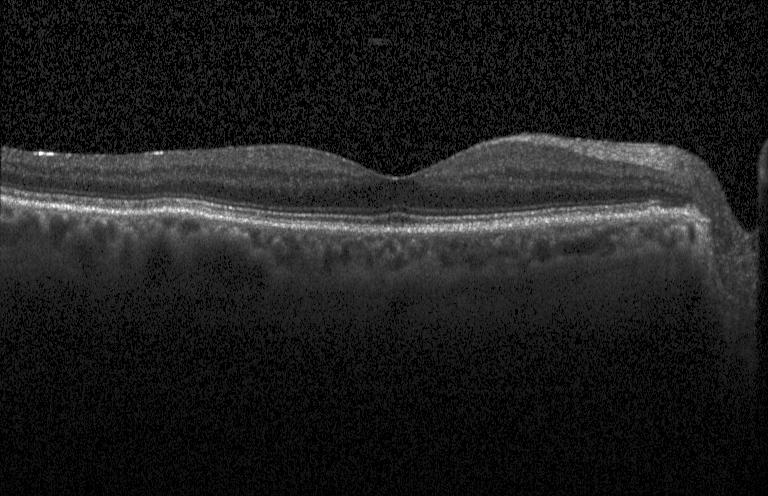
This B-scan demonstrates no CNV, no DME, and no drusen.